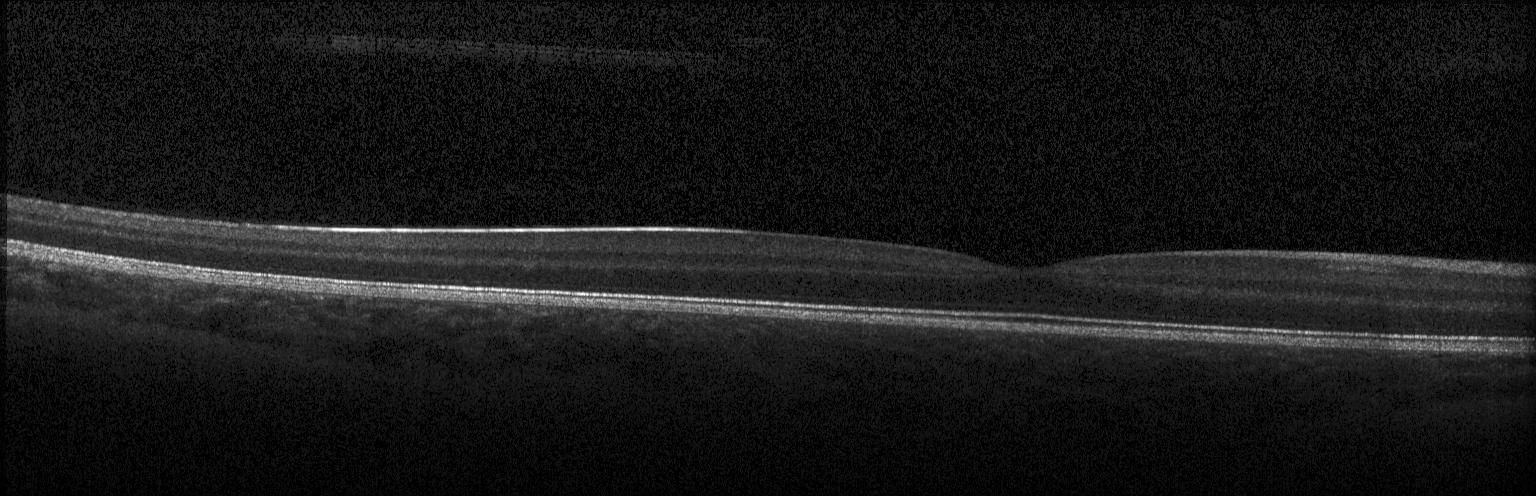 Heidelberg Spectralis, macular scan, optical coherence tomography B-scan, SD-OCT — Macular OCT: no CNV, DME, or drusen.